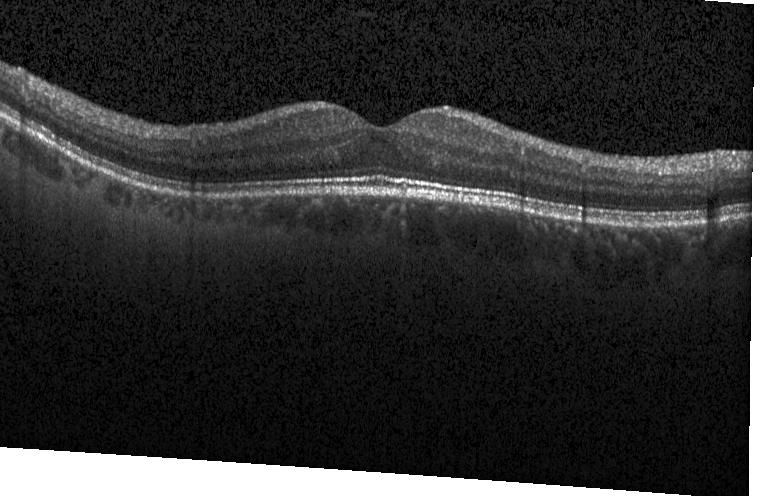
OCT B-scan; spectral-domain OCT. Diagnosis: no evidence of choroidal neovascularization, diabetic macular edema, or drusen.